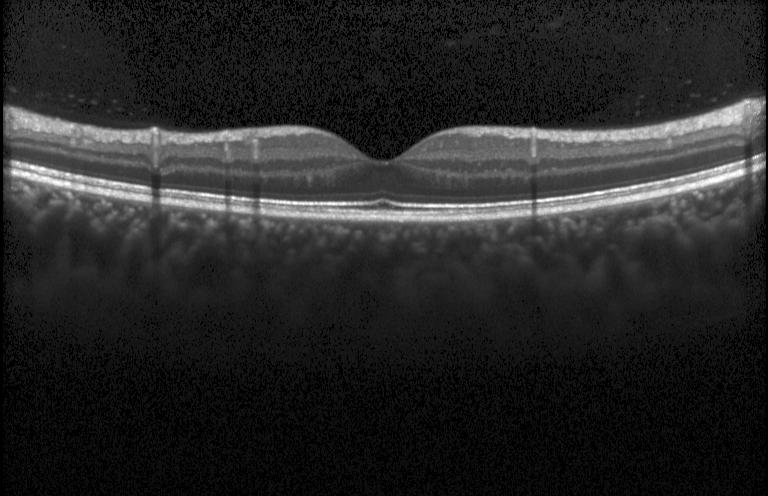

Retinal OCT cross-section. Macular OCT: no choroidal neovascularization, no diabetic macular edema, and no drusen.